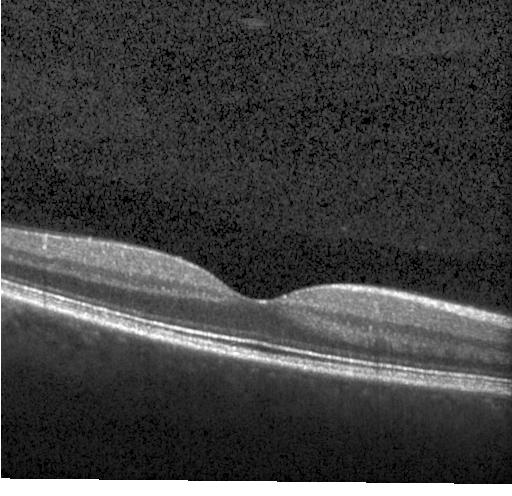

Optical coherence tomography scan. Instrument: Heidelberg Spectralis. Impression: neither choroidal neovascularization, diabetic macular edema, nor drusen.